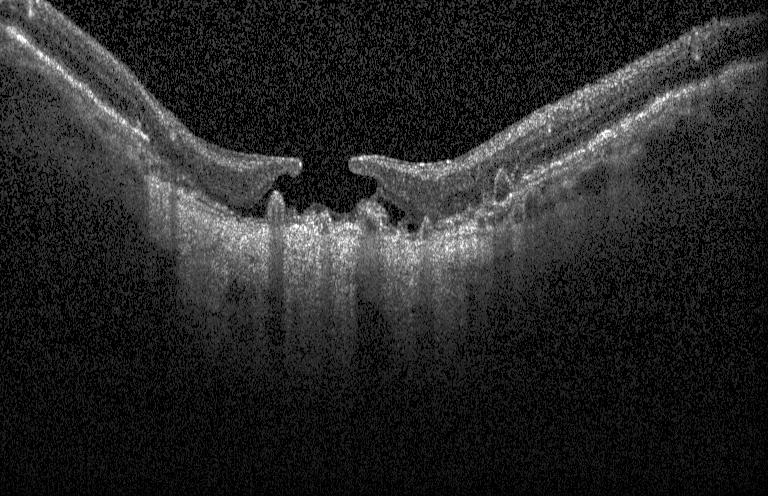 Impression: a choroidal neovascular membrane.